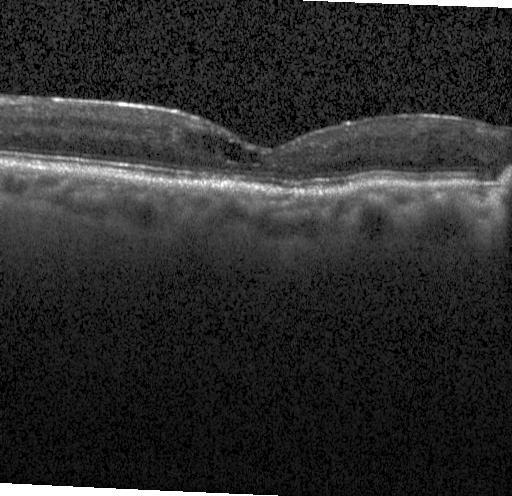 Retinal OCT B-scan; acquired on a Heidelberg Spectralis; centered on the fovea
This B-scan demonstrates DME.